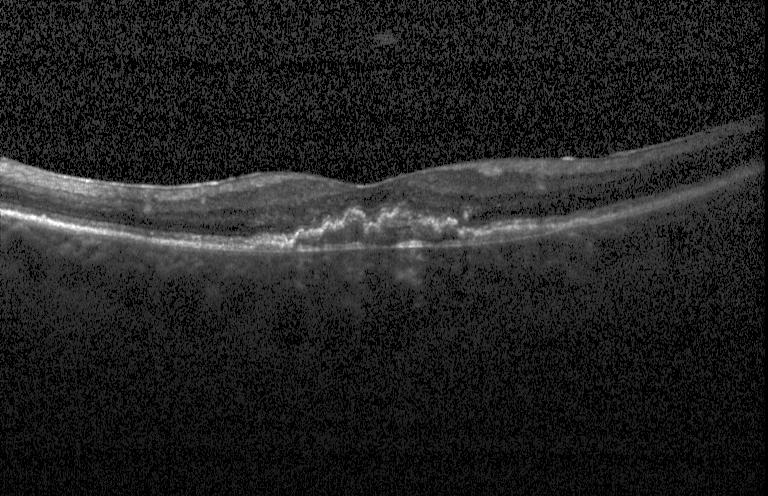
Spectral-domain optical coherence tomography; OCT line scan
Diagnosis: choroidal neovascularization (CNV).